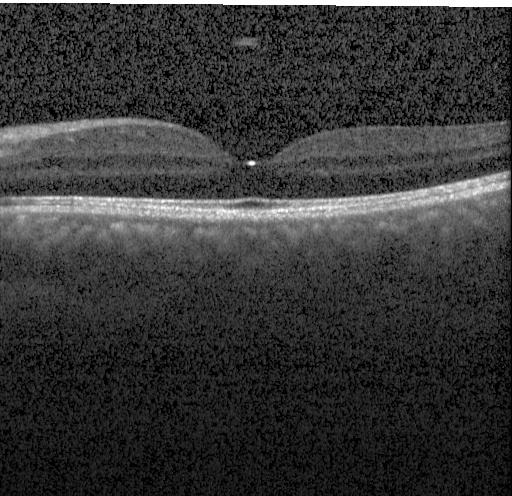

Impression: no evidence of choroidal neovascularization, diabetic macular edema, or drusen.